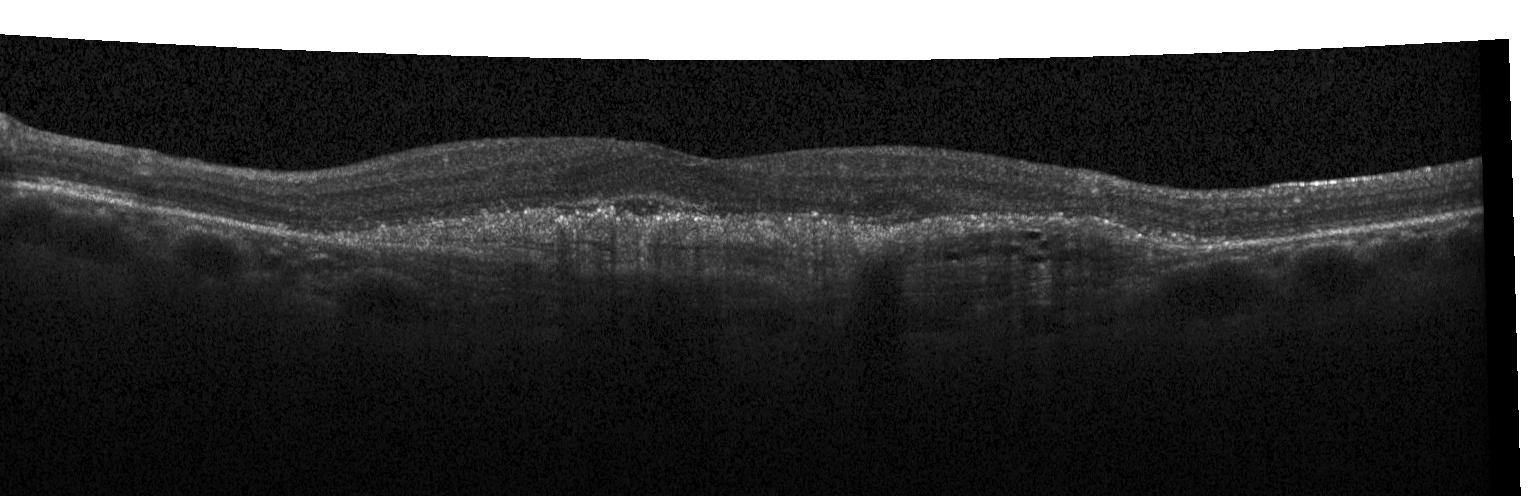
Spectral-domain OCT B-scan: a choroidal neovascular membrane.